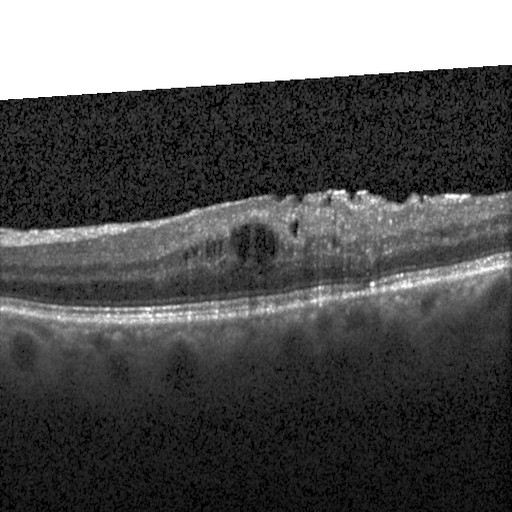 SD-OCT, acquired on a Heidelberg Spectralis, OCT line scan. Assessment: diabetic macular edema (DME).